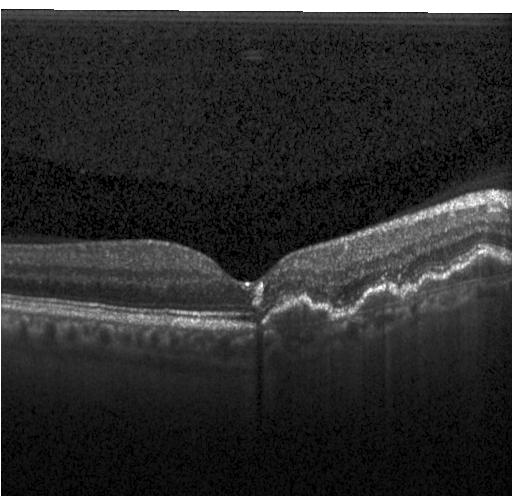

CNV.